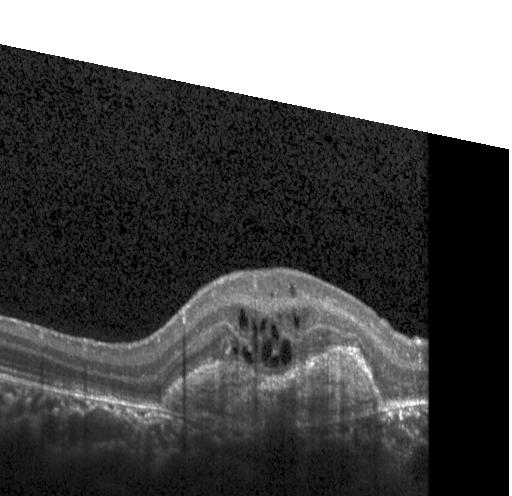

Diagnosis: a choroidal neovascular membrane.